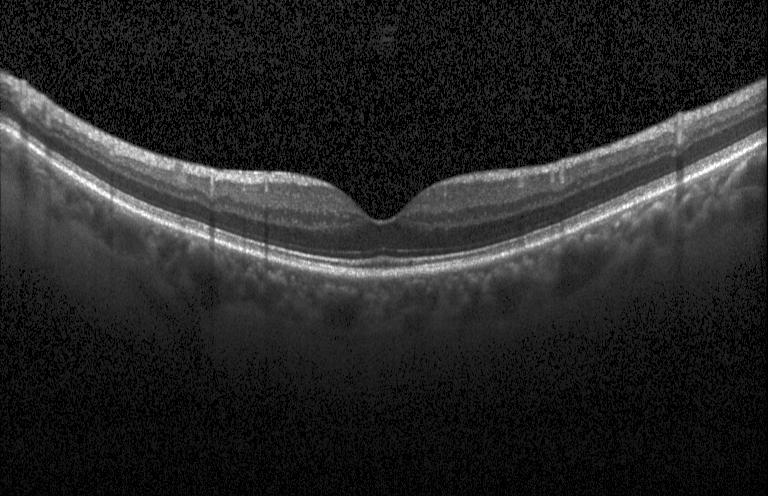
Macular OCT: no choroidal neovascularization, no diabetic macular edema, and no drusen.